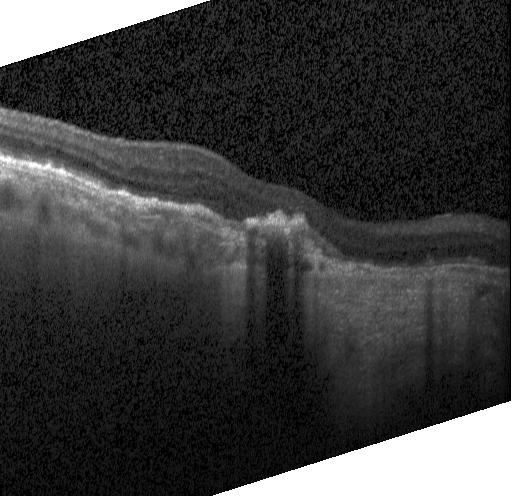

Finding: a choroidal neovascular membrane.